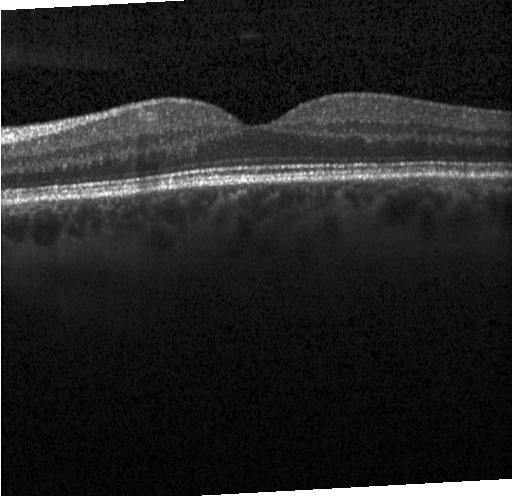

Optical coherence tomography scan — OCT finding: no choroidal neovascularization, diabetic macular edema, or drusen.